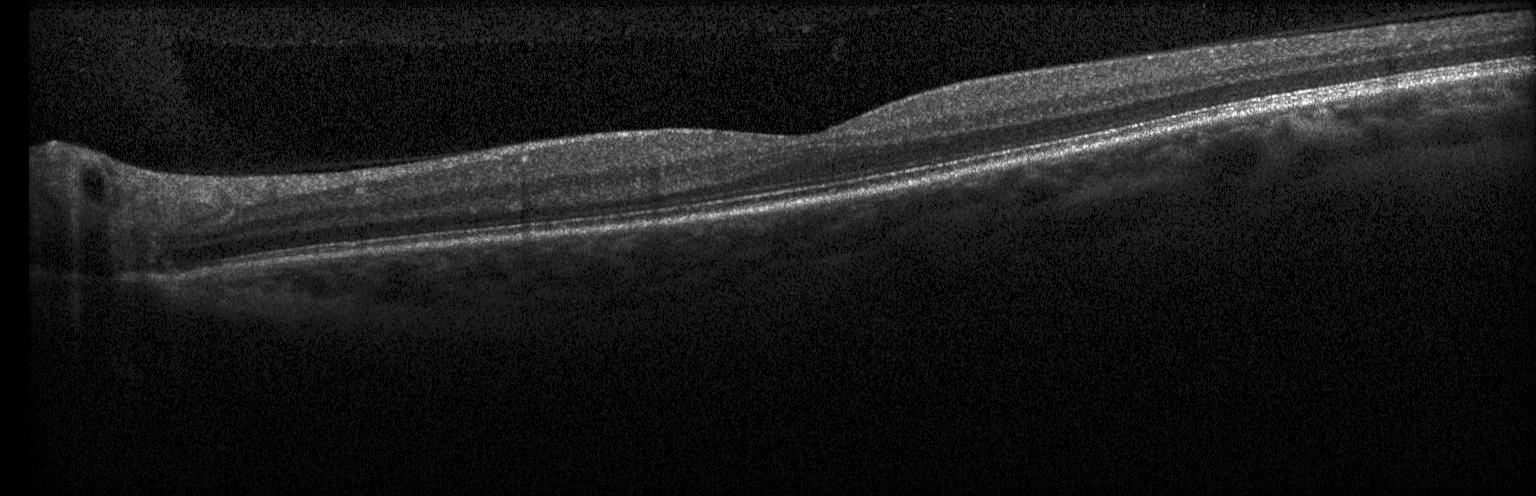
OCT line scan · spectral-domain optical coherence tomography · through the macula — The scan shows neither choroidal neovascularization, diabetic macular edema, nor drusen.